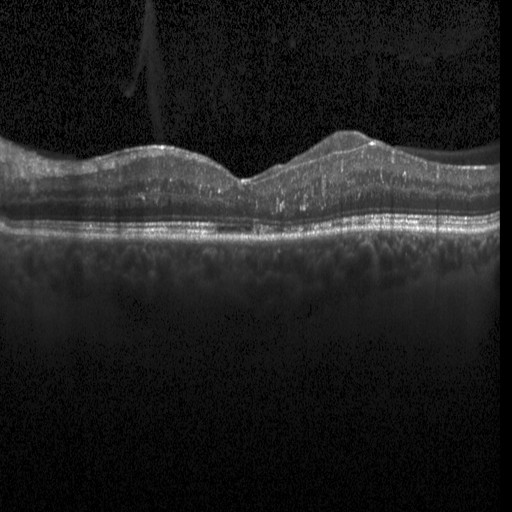

Heidelberg Spectralis, spectral-domain OCT, OCT B-scan — Diagnosis: diabetic macular edema (DME).